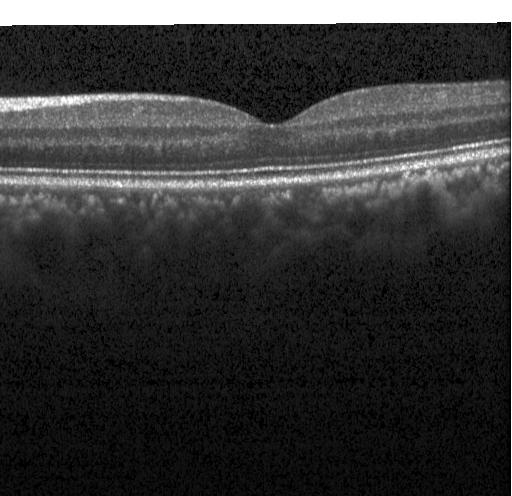

Heidelberg Spectralis OCT system, OCT line scan, SD-OCT, fovea-centered
This B-scan demonstrates no choroidal neovascularization, diabetic macular edema, or drusen.